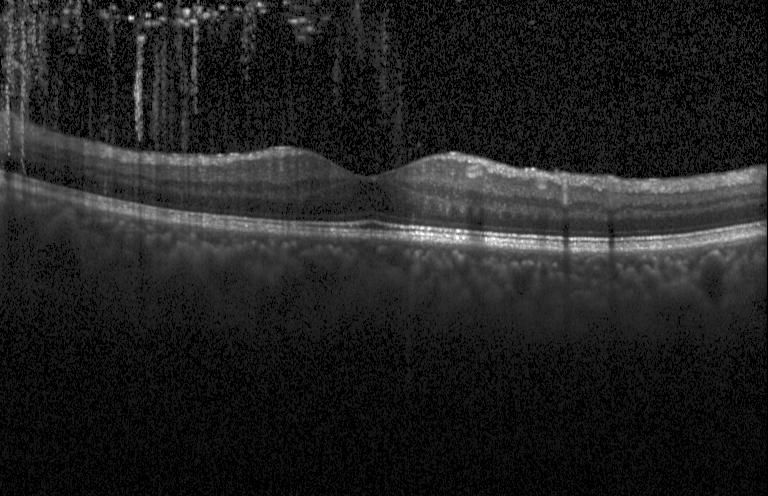 OCT B-scan showing no evidence of CNV, DME, or drusen.